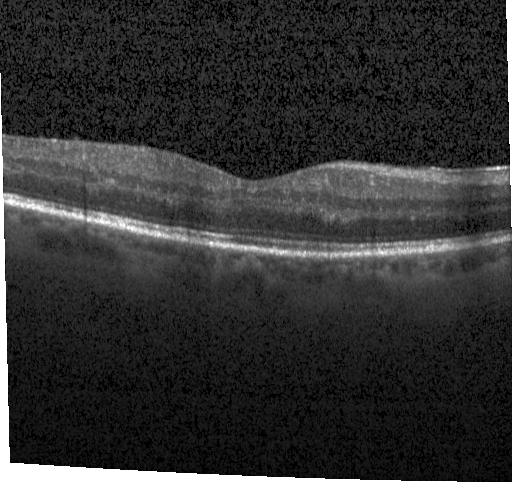 Optical coherence tomography B-scan. Finding: neither choroidal neovascularization, diabetic macular edema, nor drusen.